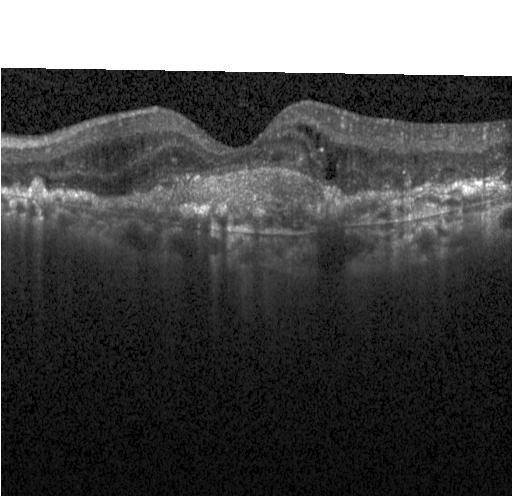

Retinal OCT B-scan, SD-OCT.
This B-scan demonstrates choroidal neovascularization (CNV).